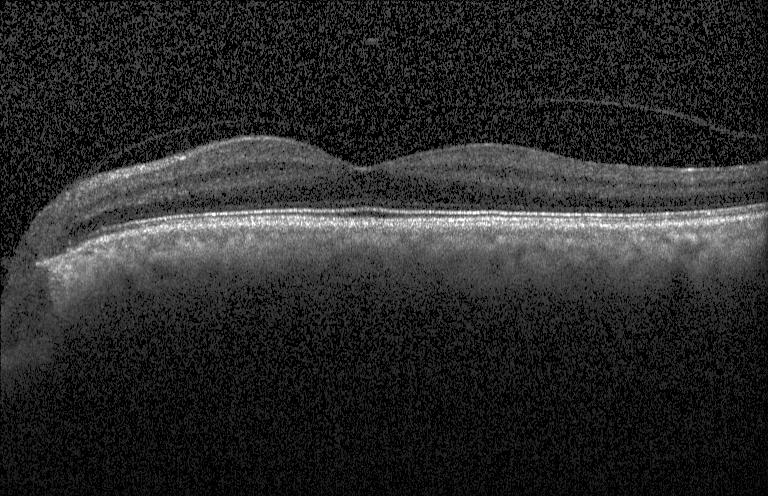 This B-scan demonstrates no choroidal neovascularization, diabetic macular edema, or drusen.